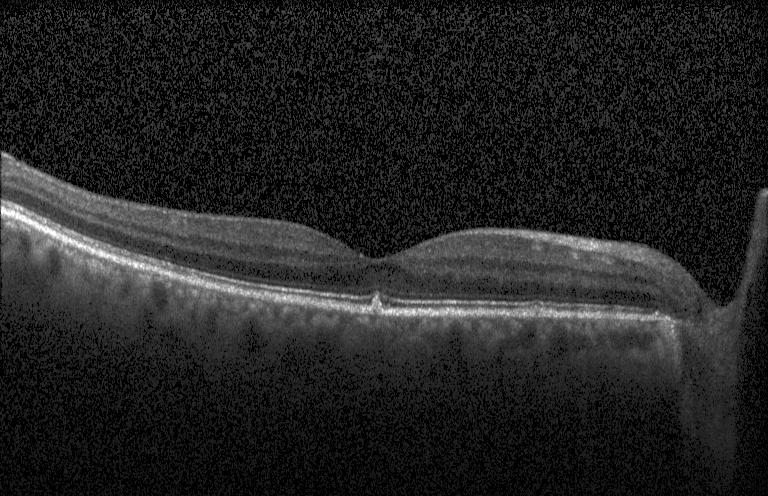

OCT finding: sub-RPE drusenoid deposits.